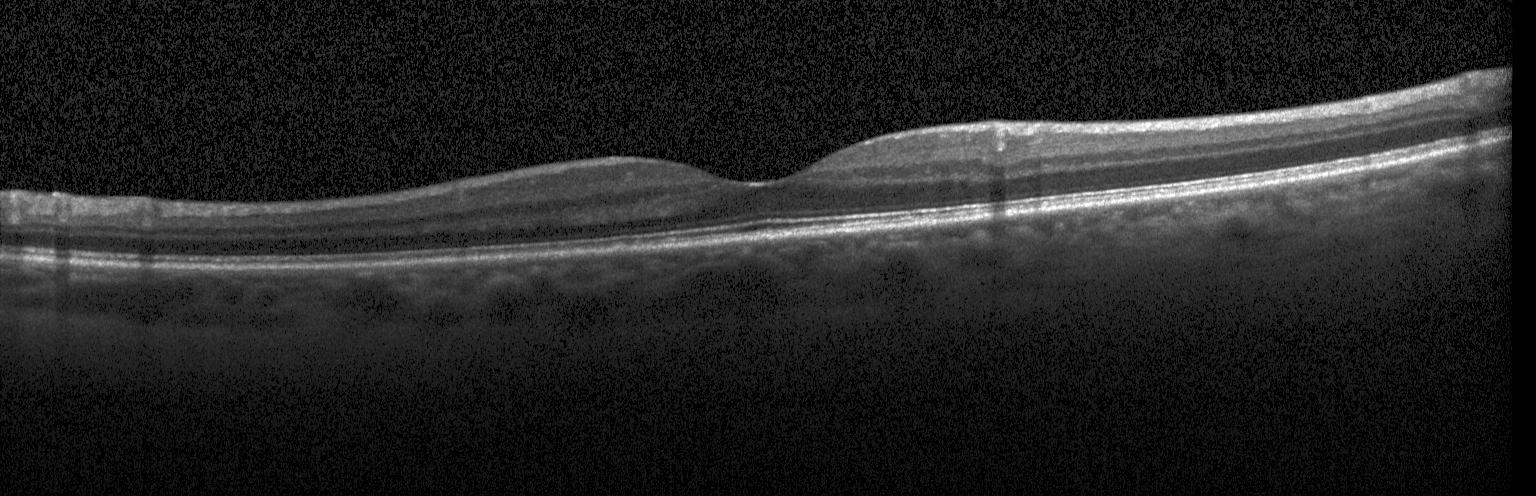 SD-OCT; optical coherence tomography scan; Heidelberg Spectralis OCT system — Macular OCT: no evidence of choroidal neovascularization, diabetic macular edema, or drusen.